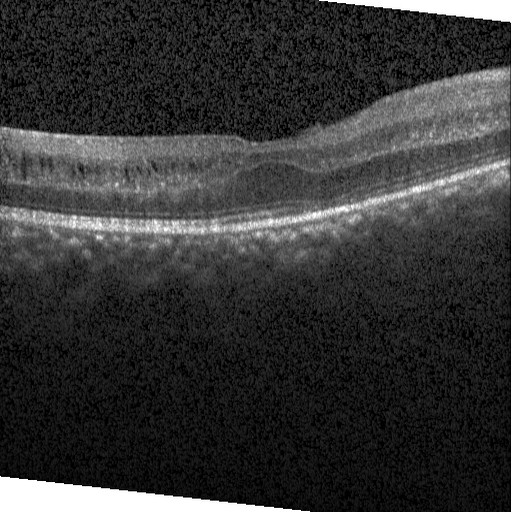
Retinal OCT cross-section showing DME.